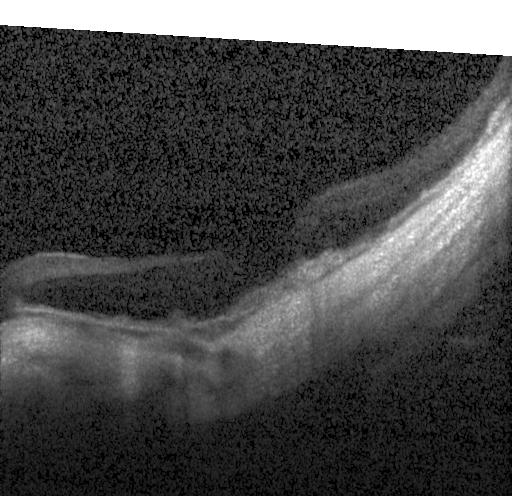 Diagnosis: CNV.